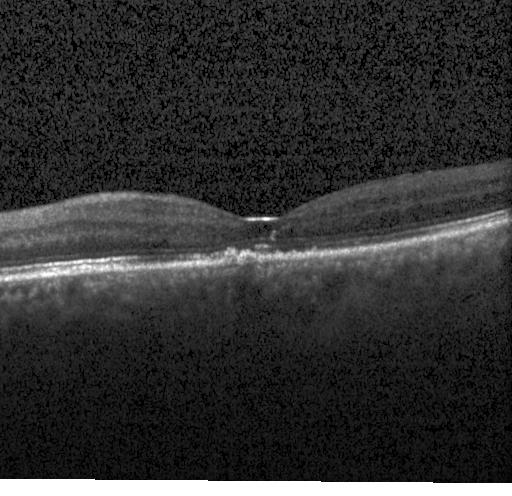

Optical coherence tomography B-scan. OCT finding: multiple drusen.